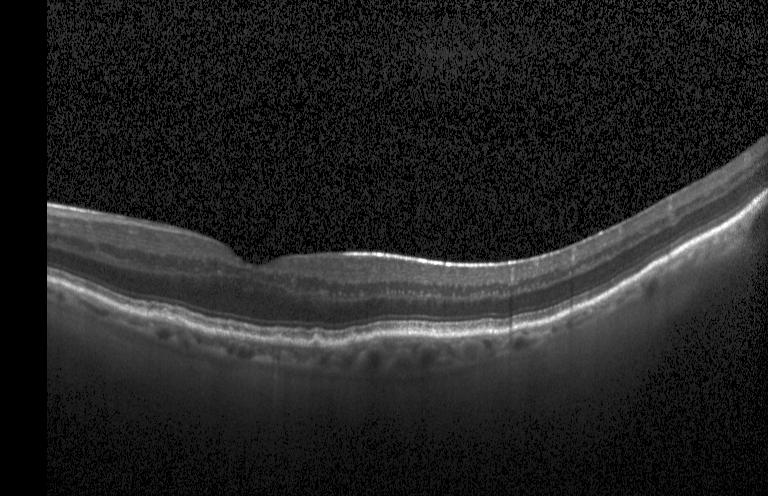
Optical coherence tomography scan; acquired on a Heidelberg Spectralis; through the macula.
Assessment: drusen.